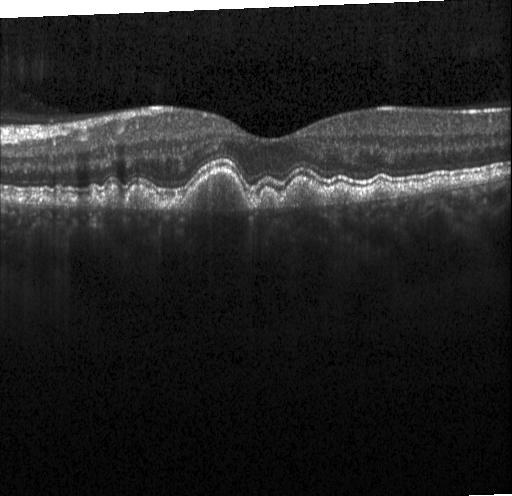 Retinal OCT cross-section · spectral-domain OCT · acquired on a Heidelberg Spectralis · through the macula
Finding: multiple drusen.